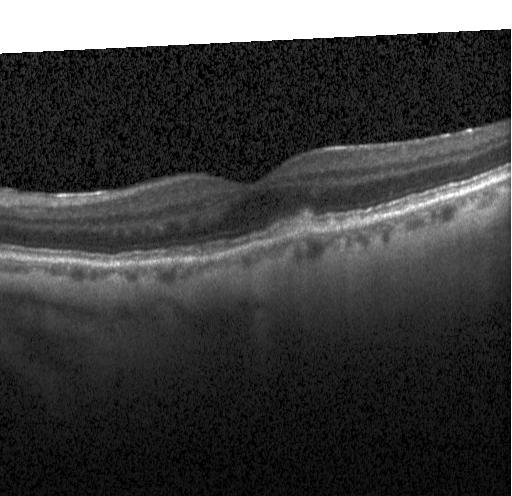

OCT line scan. Impression: drusen.